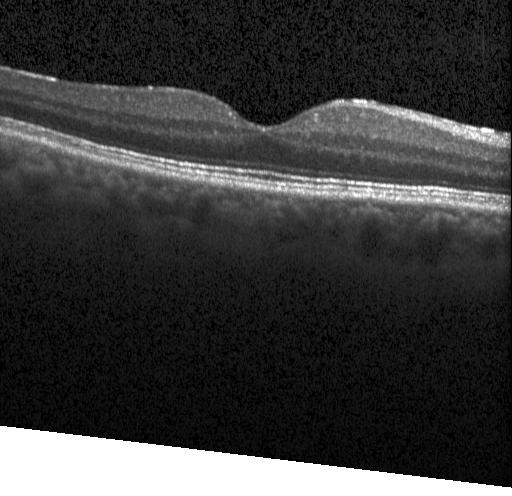 Heidelberg Spectralis · fovea-centered · spectral-domain OCT · retinal OCT cross-section — Finding: neither choroidal neovascularization, diabetic macular edema, nor drusen.